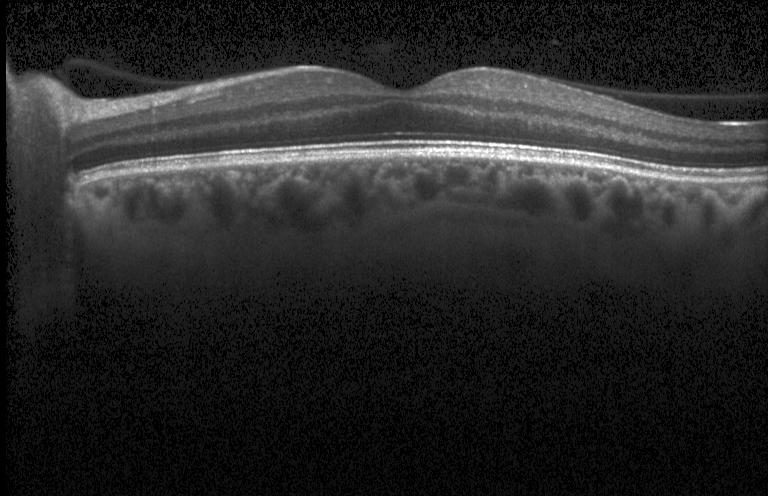
Retinal OCT B-scan; Heidelberg Spectralis OCT system. Finding: no CNV, DME, or drusen.